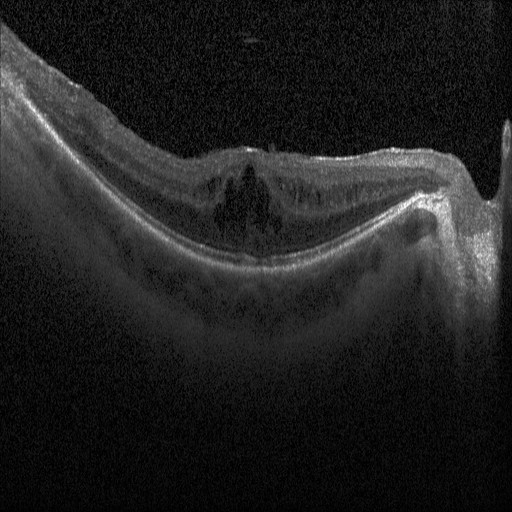

SD-OCT. Optical coherence tomography scan. Acquired on a Heidelberg Spectralis. Macular scan.
Assessment: diabetic macular edema.